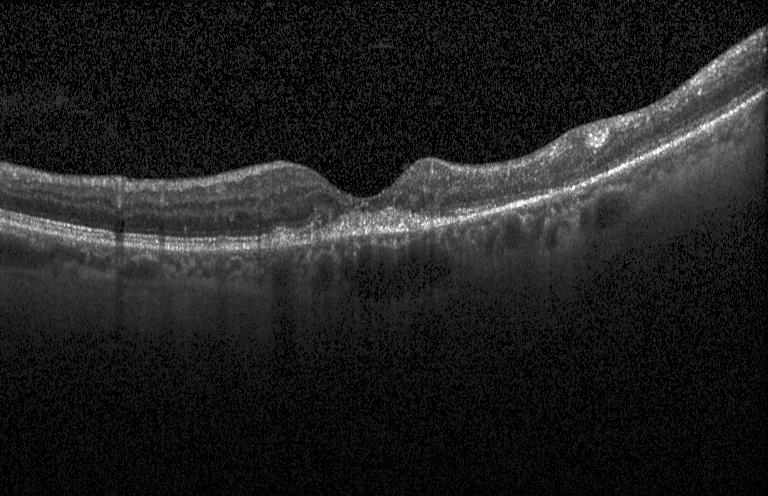

OCT finding: a choroidal neovascular membrane.